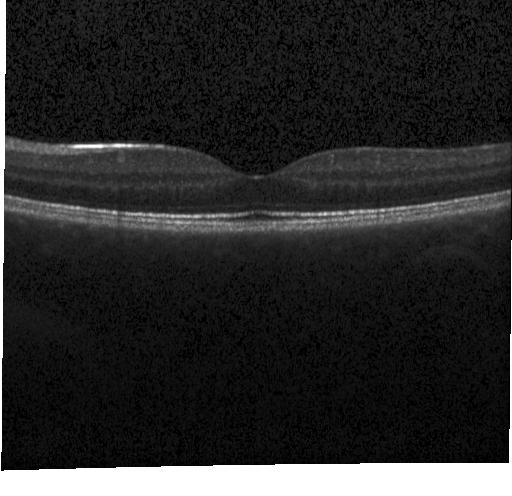

OCT B-scan; acquired on a Heidelberg Spectralis; fovea-centered; spectral-domain OCT. This B-scan demonstrates no choroidal neovascularization, no diabetic macular edema, and no drusen.